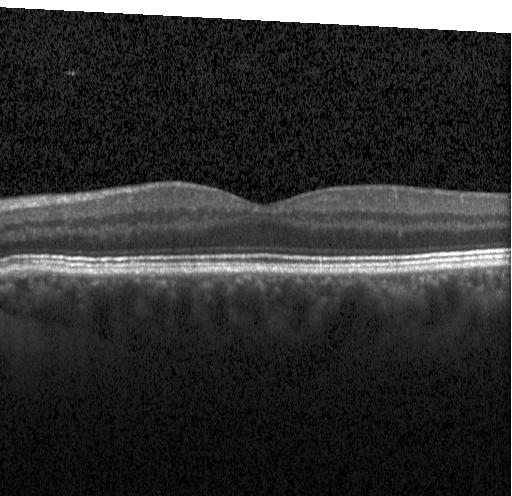

Dx: no choroidal neovascularization, diabetic macular edema, or drusen.